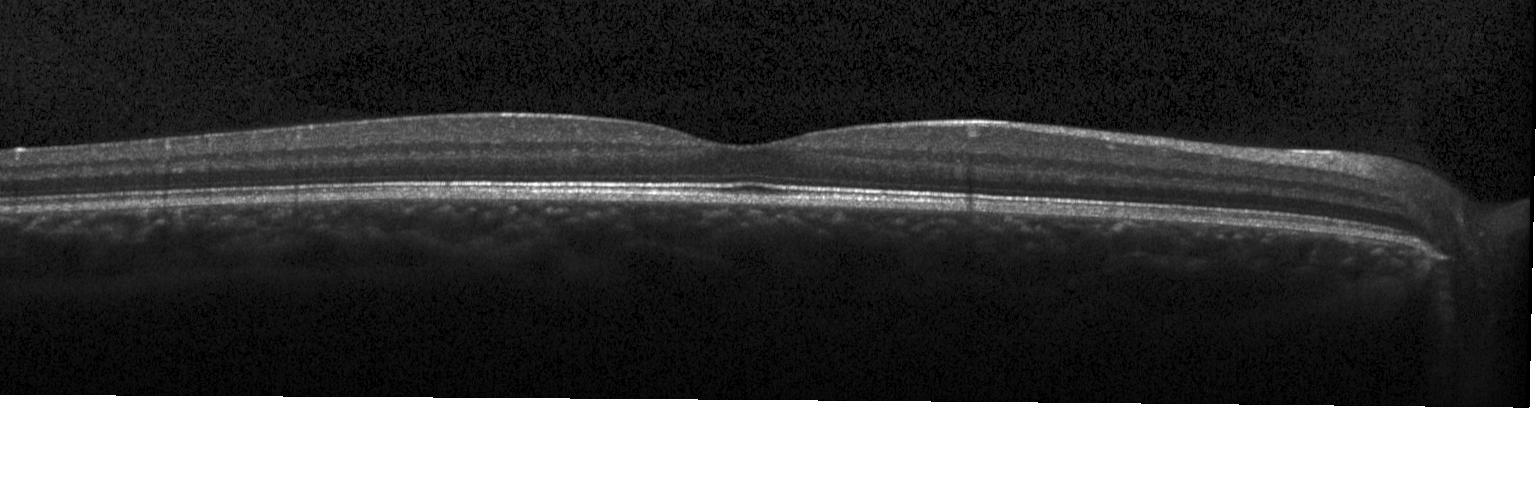
OCT B-scan — Assessment: neither CNV, DME, nor drusen.